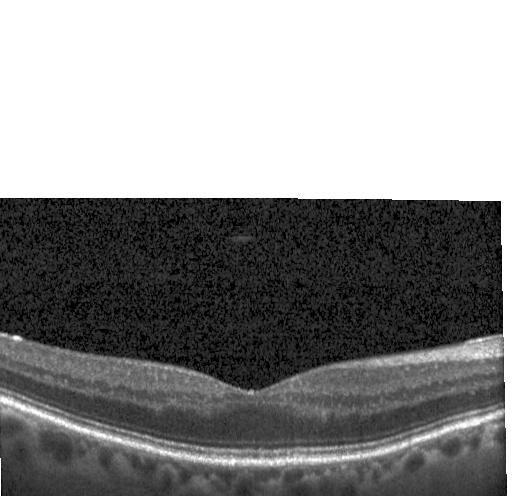 Impression: no choroidal neovascularization, diabetic macular edema, or drusen.